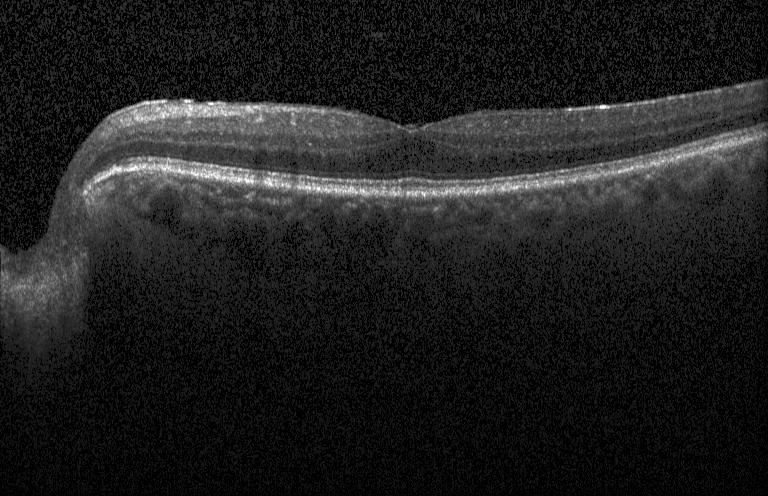 Optical coherence tomography scan, spectral-domain optical coherence tomography — Diagnosis: no evidence of CNV, DME, or drusen.